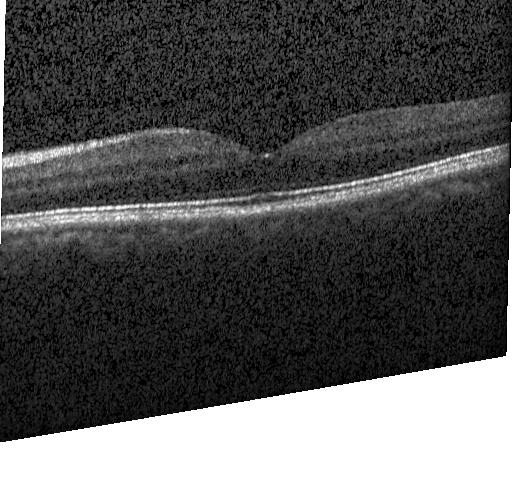
Heidelberg Spectralis; fovea-centered; retinal OCT cross-section; spectral-domain OCT — Diagnosis: no CNV, no DME, and no drusen.